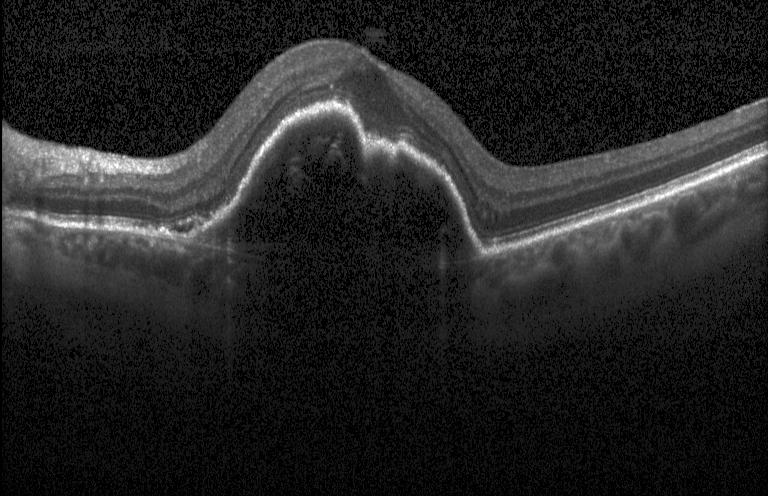 OCT finding: a choroidal neovascular membrane.